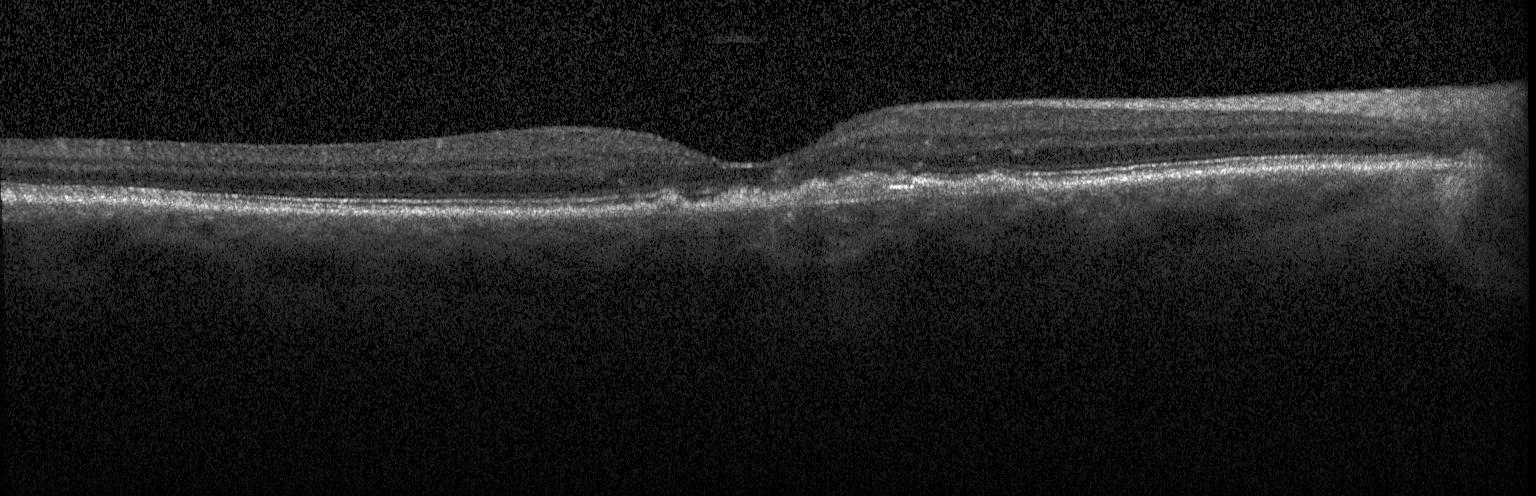 Optical coherence tomography B-scan, through the macula, Heidelberg Spectralis OCT system.
Finding: CNV.